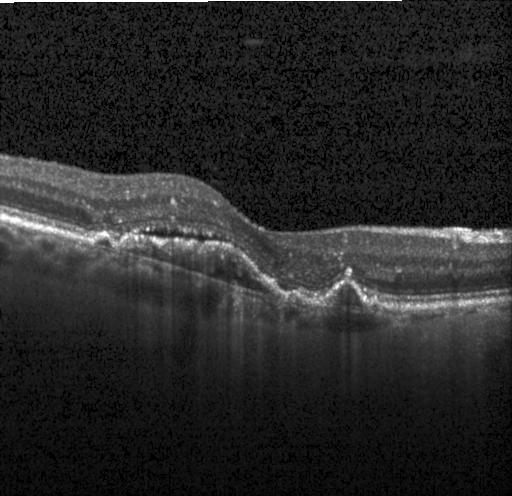 Retinal OCT cross-section. Assessment: a choroidal neovascular membrane.